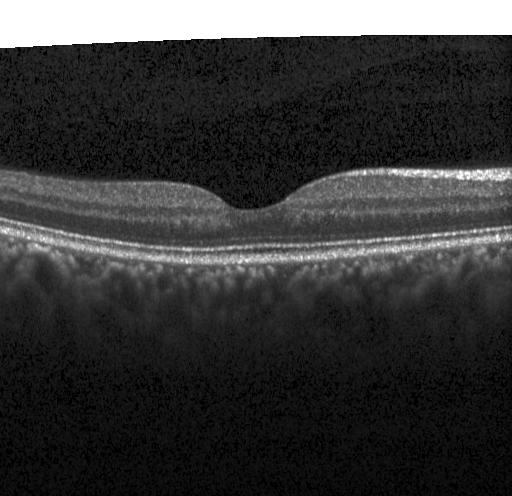 Spectral-domain OCT · retinal OCT B-scan · acquired on a Heidelberg Spectralis
Macular OCT: no CNV, no DME, and no drusen.